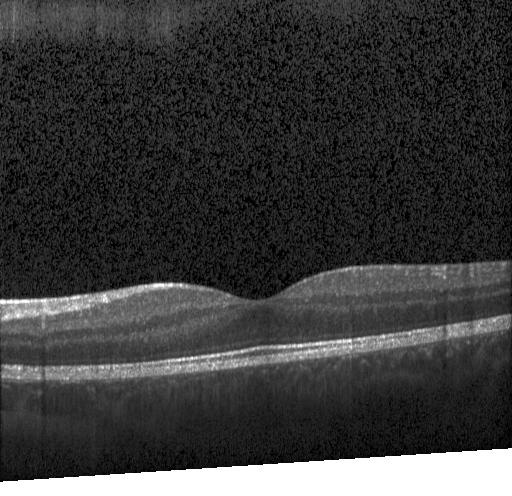 This B-scan demonstrates neither choroidal neovascularization, diabetic macular edema, nor drusen.